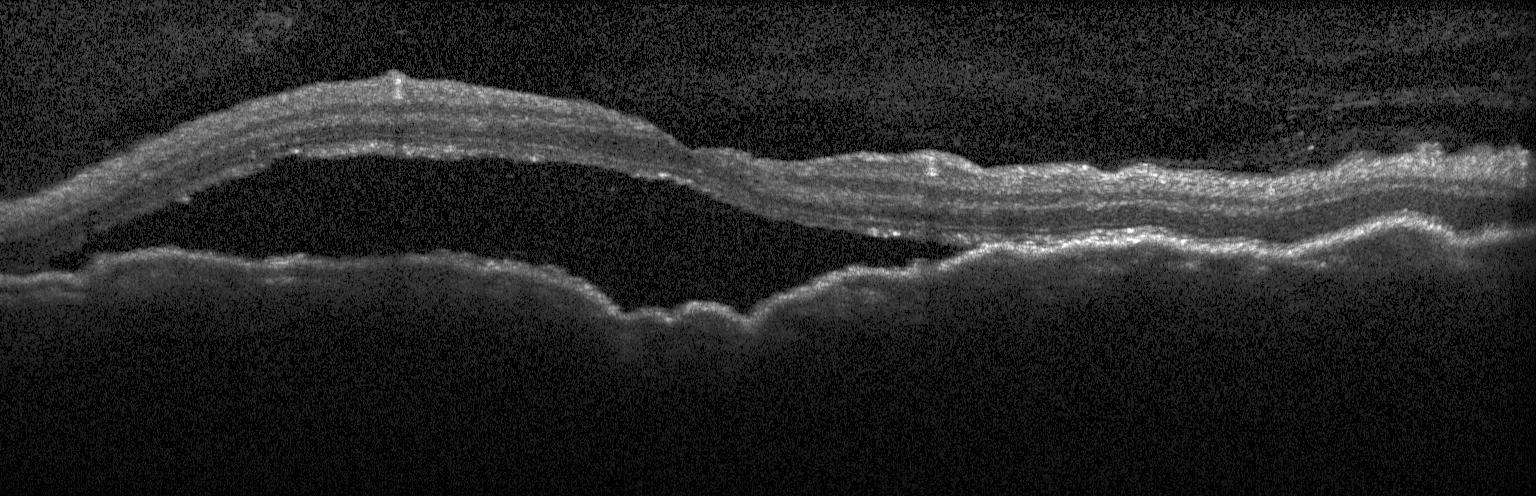
Finding: choroidal neovascularization.